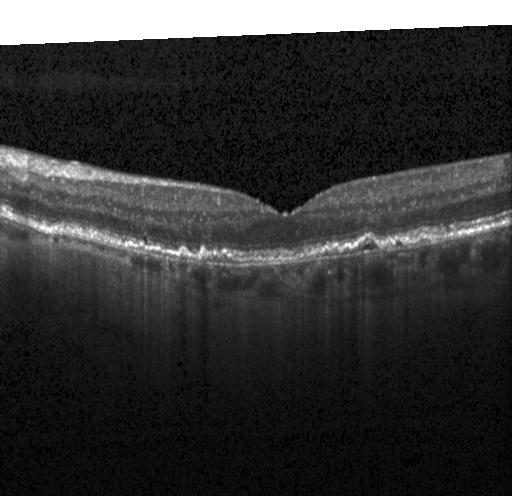

Spectral-domain OCT · Heidelberg Spectralis · optical coherence tomography B-scan — Macular OCT: multiple drusen.